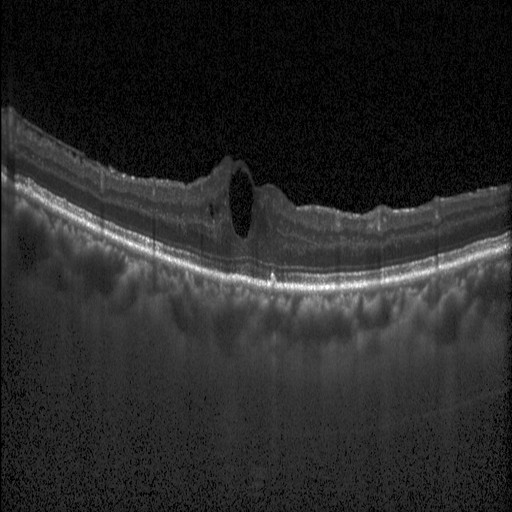

OCT finding: diabetic macular edema.